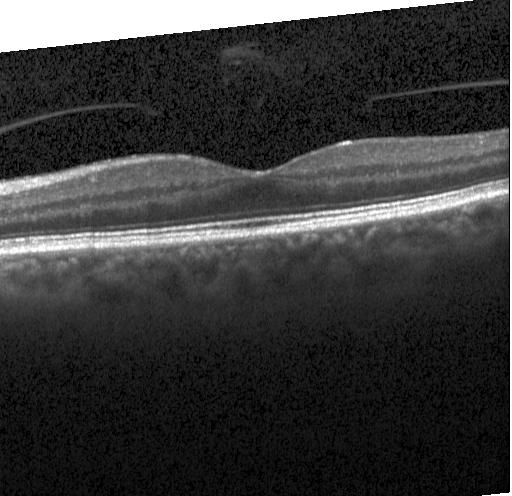

This B-scan demonstrates no evidence of choroidal neovascularization, diabetic macular edema, or drusen.